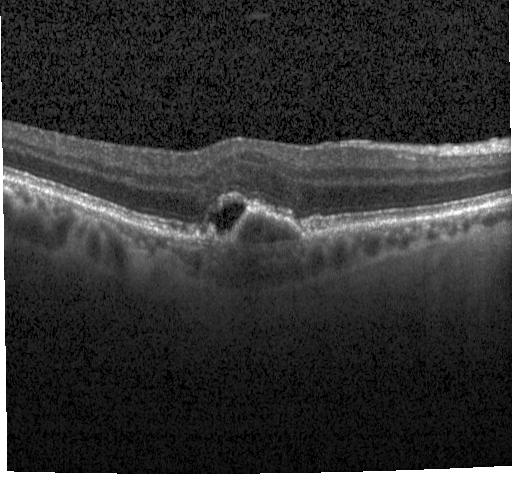 Acquired on a Heidelberg Spectralis. Centered on the fovea. OCT line scan. Diagnosis: CNV.